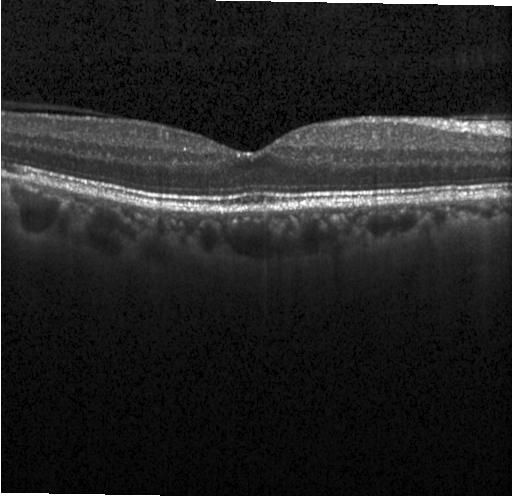

OCT line scan — Impression: neither choroidal neovascularization, diabetic macular edema, nor drusen.